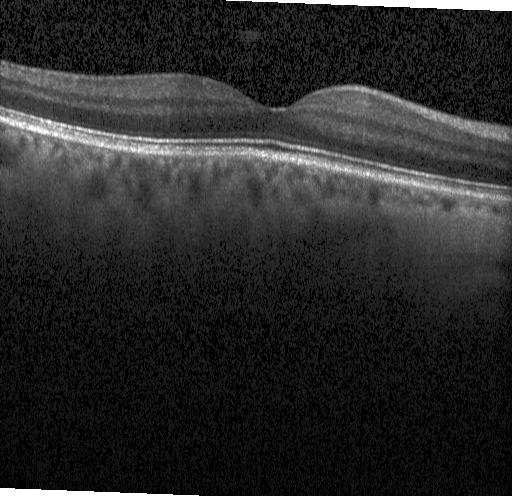
Macular OCT demonstrating no choroidal neovascularization, diabetic macular edema, or drusen.